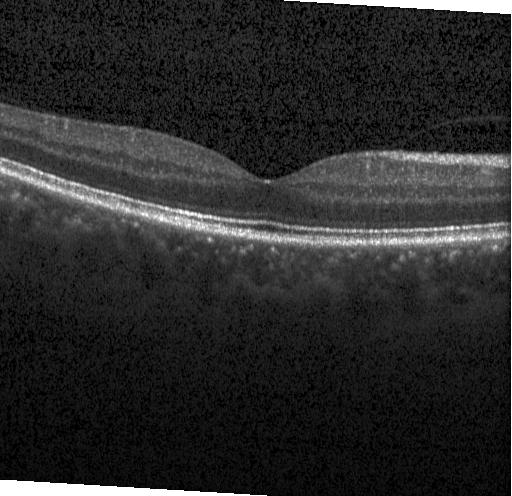 OCT B-scan · centered on the fovea · instrument: Heidelberg Spectralis · spectral-domain OCT.
Assessment: no CNV, no DME, and no drusen.